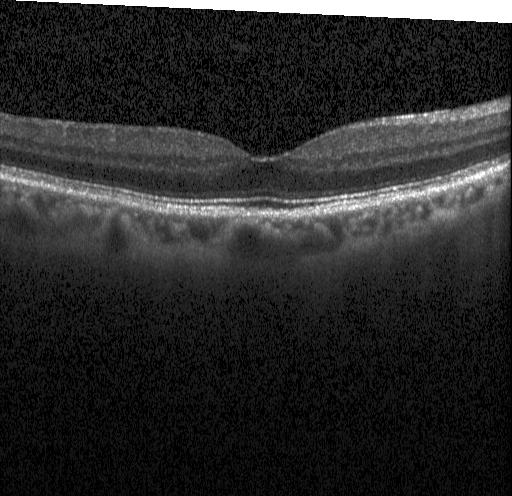

Optical coherence tomography B-scan, fovea-centered. Dx: no evidence of choroidal neovascularization, diabetic macular edema, or drusen.